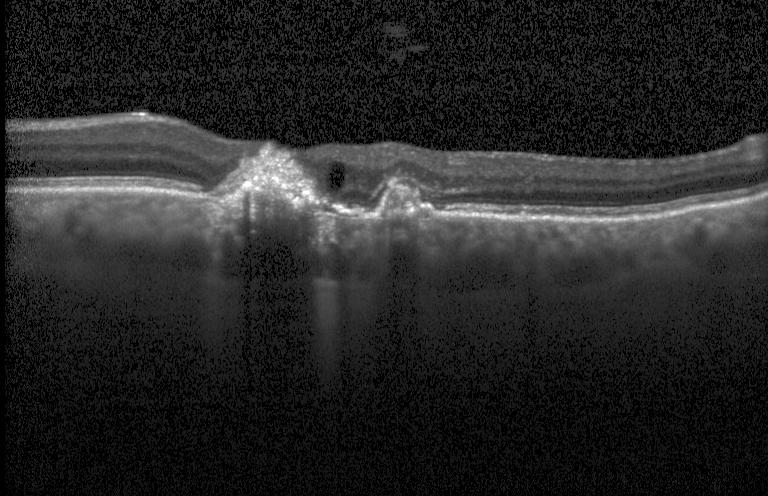
Retinal OCT B-scan
Finding: a choroidal neovascular membrane.